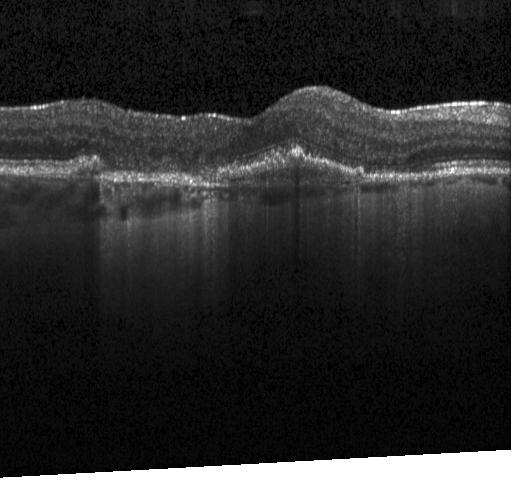 OCT line scan; spectral-domain OCT; Heidelberg Spectralis OCT system; fovea-centered
The scan shows a choroidal neovascular membrane.